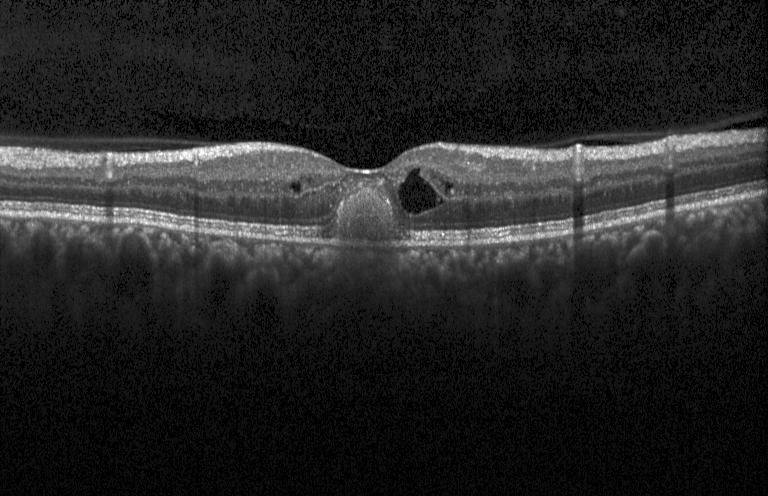
Macular scan · spectral-domain optical coherence tomography · optical coherence tomography scan · instrument: Heidelberg Spectralis. A choroidal neovascular membrane.